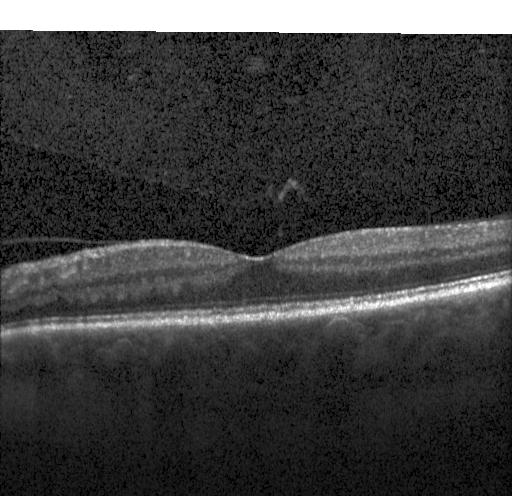 Diagnosis: neither CNV, DME, nor drusen.